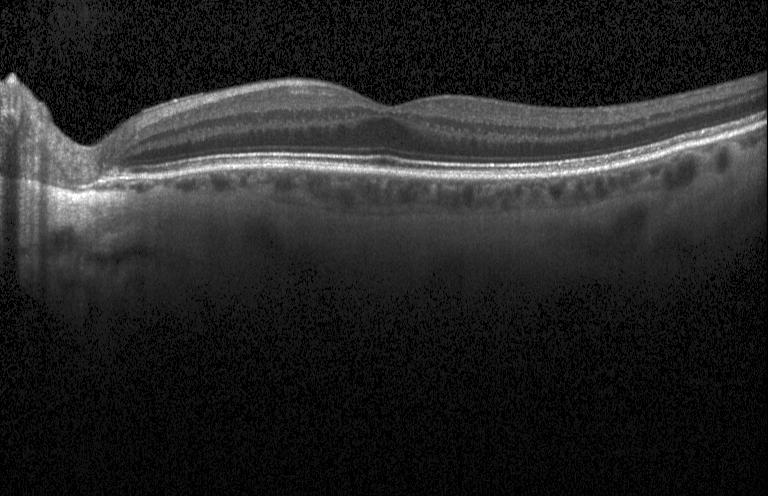

OCT finding: no CNV, DME, or drusen.